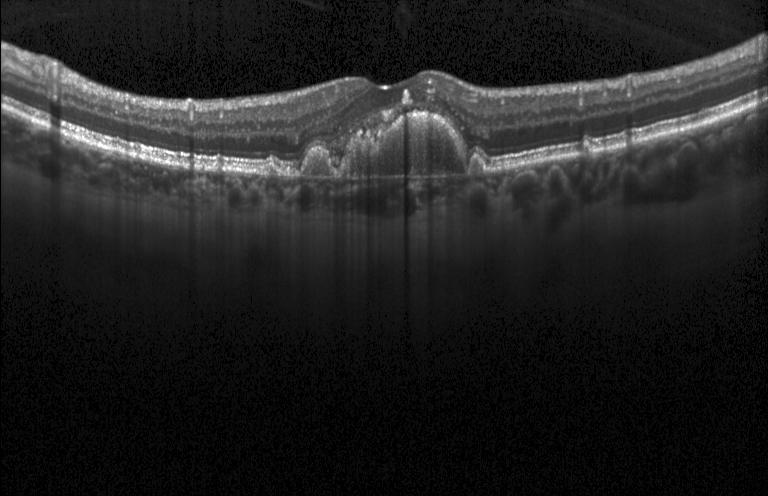

Impression: a choroidal neovascular membrane.